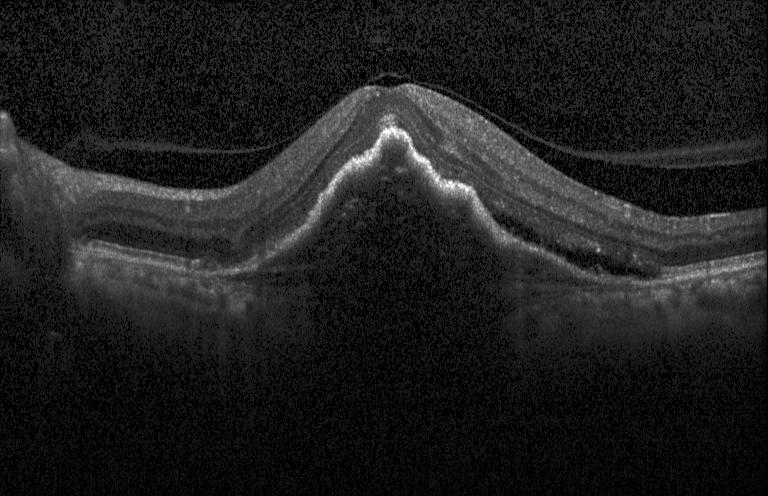
Heidelberg Spectralis OCT system · retinal OCT cross-section · fovea-centered · spectral-domain OCT
This B-scan demonstrates a choroidal neovascular membrane.